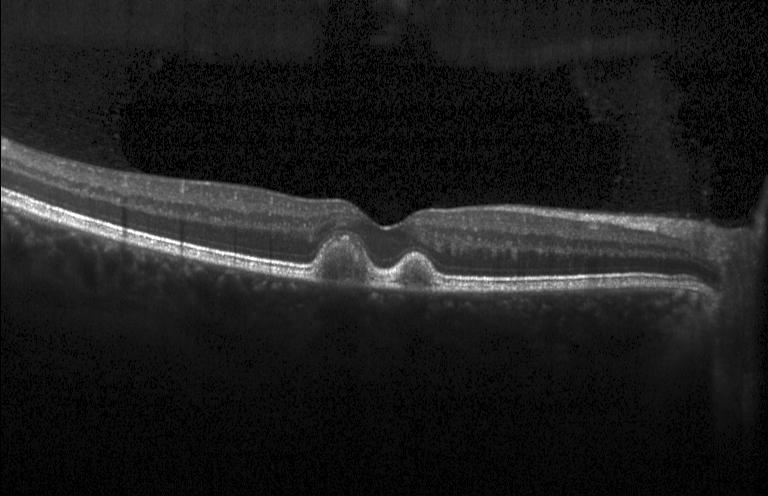
Spectral-domain OCT. Retinal OCT B-scan. Through the macula
Dx: sub-RPE drusenoid deposits.